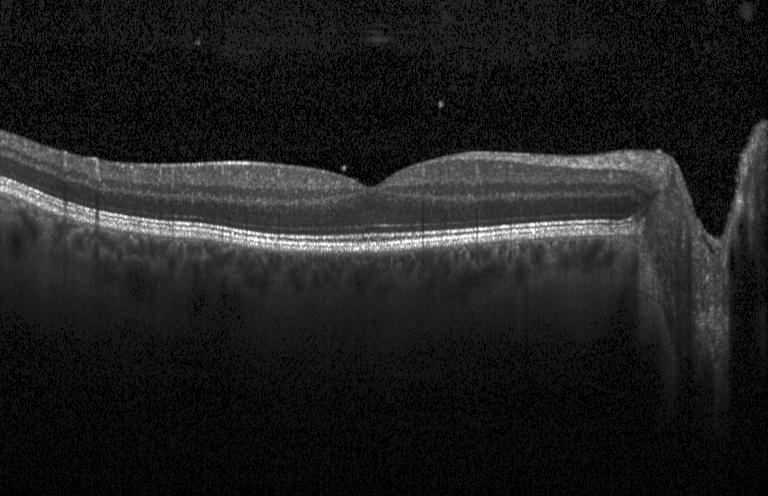 Finding: no evidence of CNV, DME, or drusen.